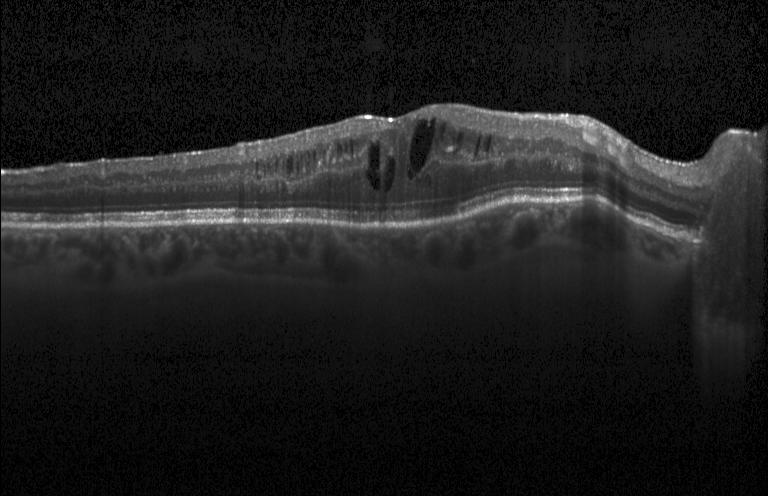
OCT B-scan, SD-OCT. Diagnosis: diabetic macular edema (DME).